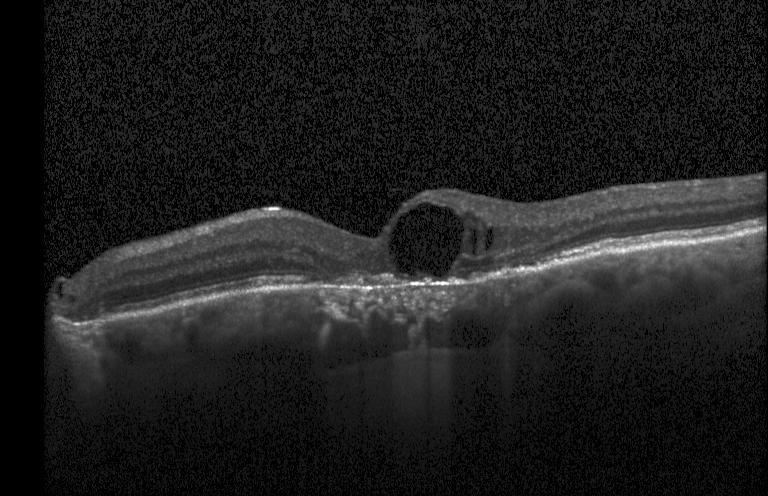
Through the macula. Retinal OCT B-scan — Finding: choroidal neovascularization (CNV).